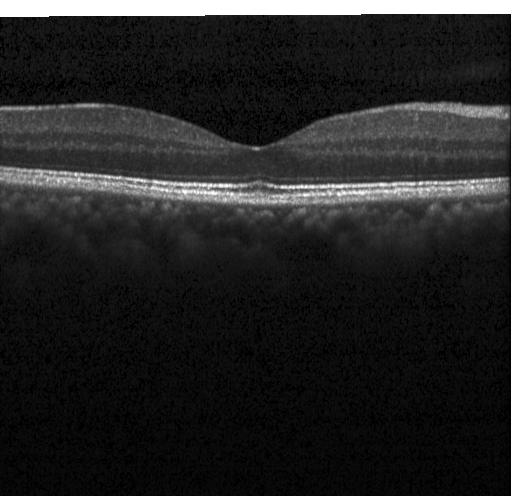 Instrument: Heidelberg Spectralis · optical coherence tomography scan · spectral-domain optical coherence tomography · centered on the fovea
Diagnosis: no evidence of choroidal neovascularization, diabetic macular edema, or drusen.